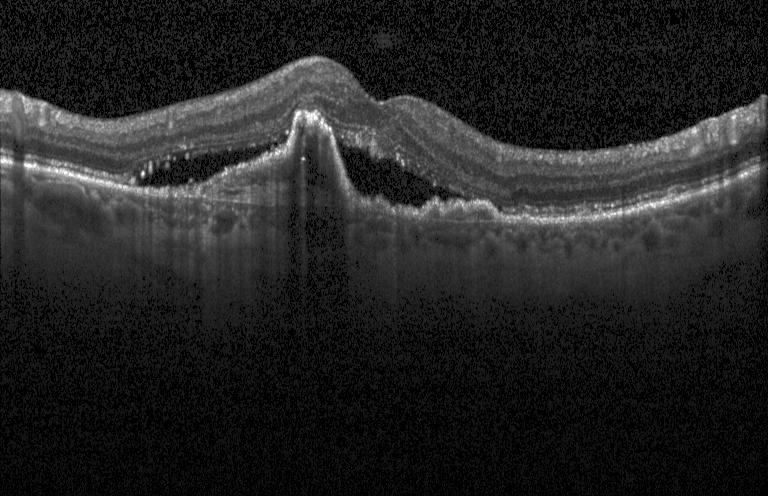
Spectral-domain optical coherence tomography, OCT line scan, through the macula, acquired on a Heidelberg Spectralis
Impression: a choroidal neovascular membrane.